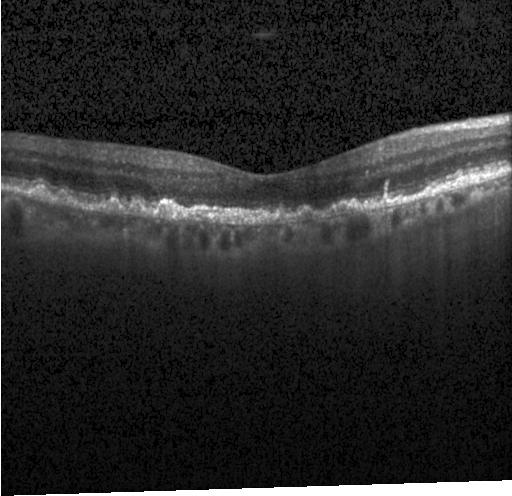

Centered on the fovea, acquired on a Heidelberg Spectralis, SD-OCT, optical coherence tomography scan.
Dx: a choroidal neovascular membrane.